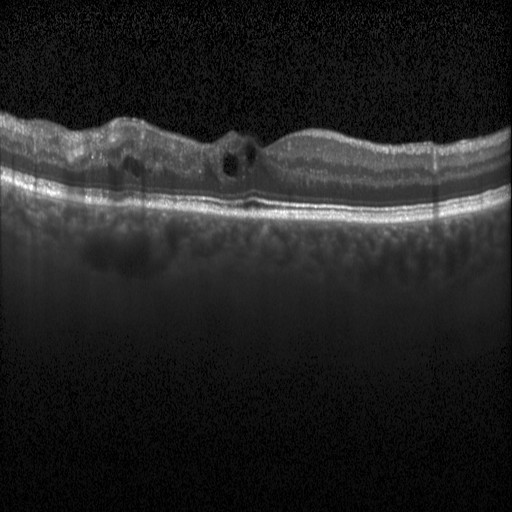
Macular OCT demonstrating diabetic macular edema (DME).